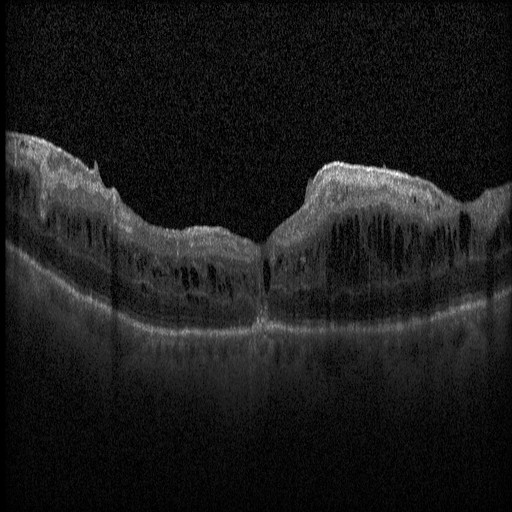

Heidelberg Spectralis OCT system. Spectral-domain optical coherence tomography. Macular scan. OCT line scan. Diagnosis: diabetic macular edema (DME).